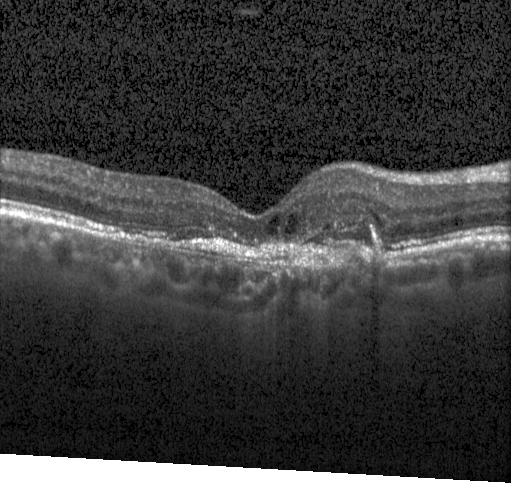
Diagnosis: choroidal neovascularization.